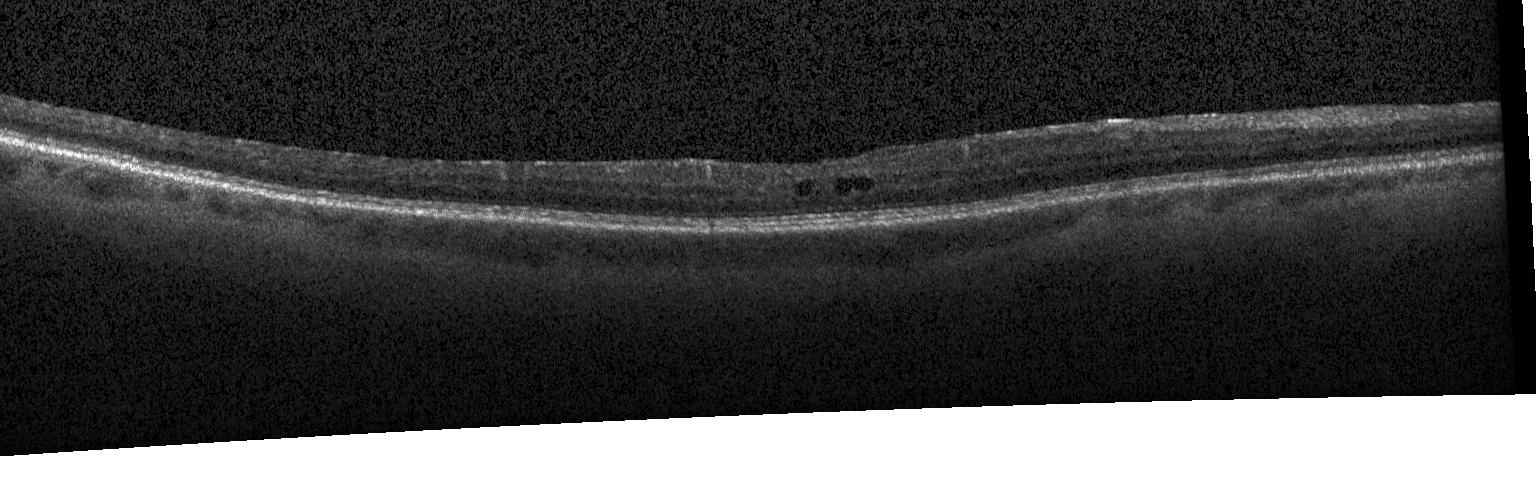 OCT finding: DME.